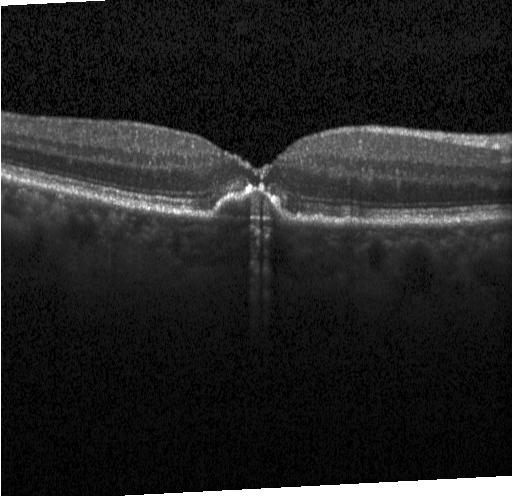 Spectral-domain optical coherence tomography · through the macula · OCT B-scan · acquired on a Heidelberg Spectralis.
Diagnosis: a choroidal neovascular membrane.